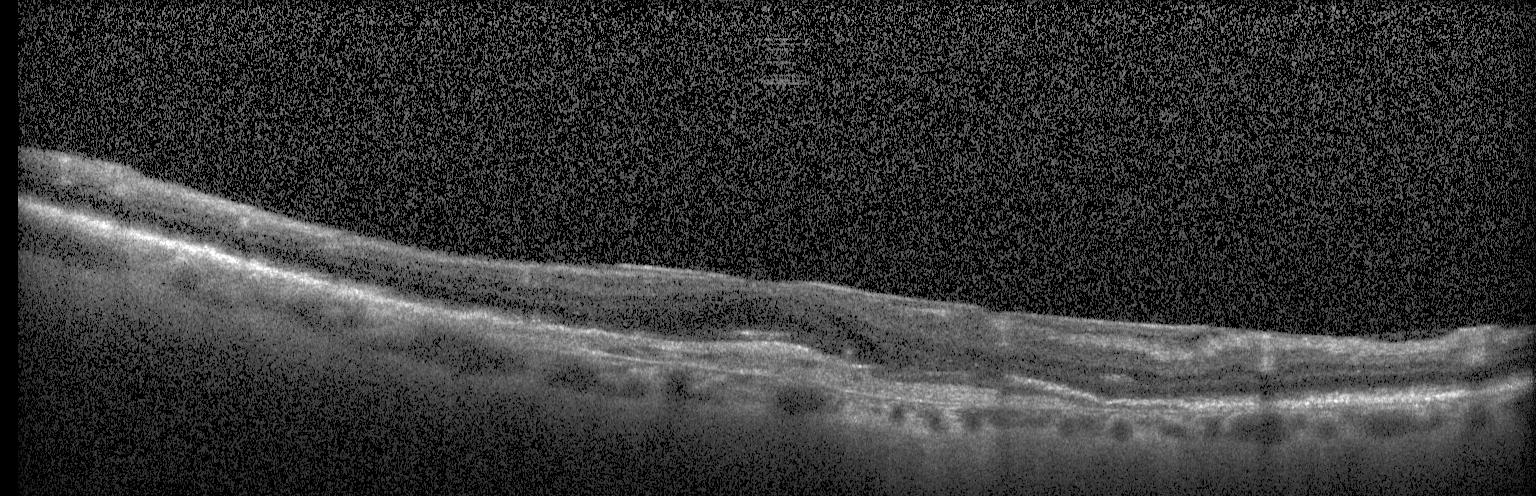

The scan shows a choroidal neovascular membrane.